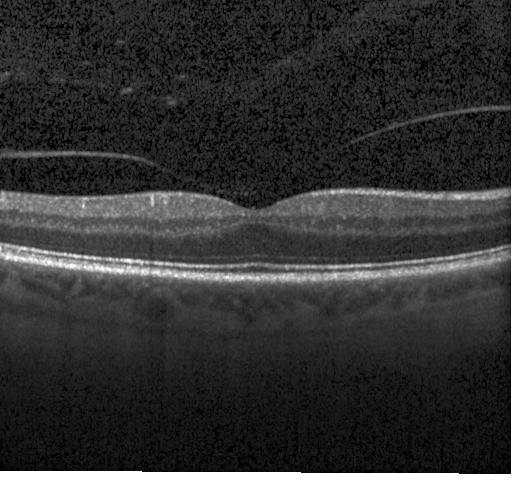

OCT scan showing no CNV, no DME, and no drusen.